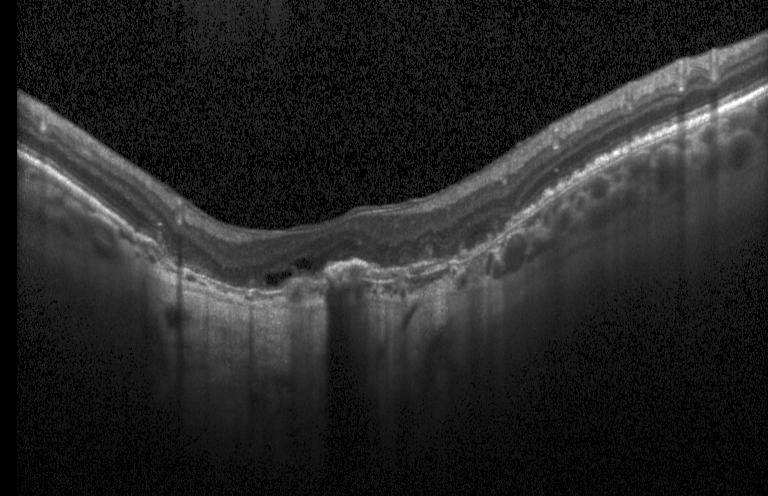

Macular OCT: a choroidal neovascular membrane.